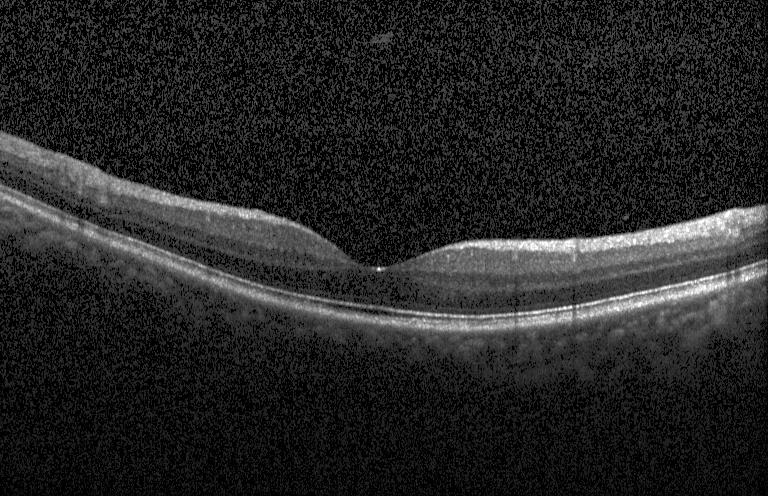
Optical coherence tomography scan · spectral-domain optical coherence tomography · Heidelberg Spectralis.
Diagnosis: no evidence of choroidal neovascularization, diabetic macular edema, or drusen.